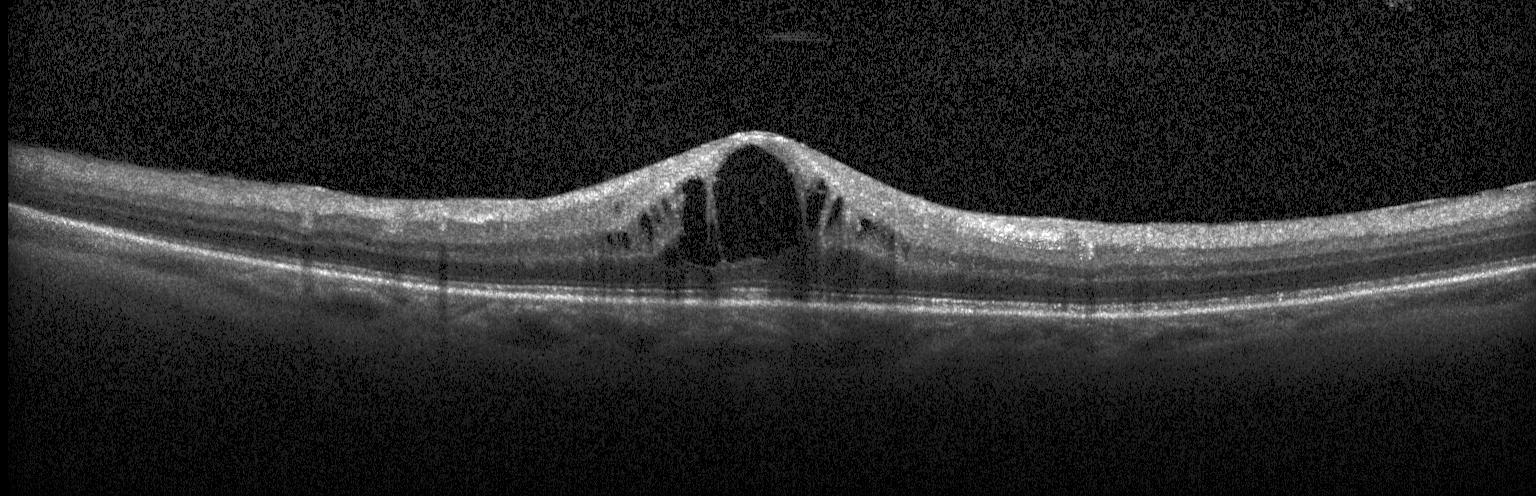
Heidelberg Spectralis OCT system. Macular scan. Retinal OCT cross-section
Impression: diabetic macular edema.